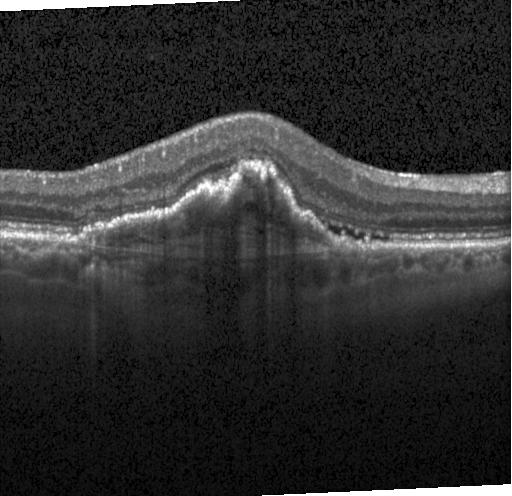
Spectral-domain OCT B-scan: a choroidal neovascular membrane.